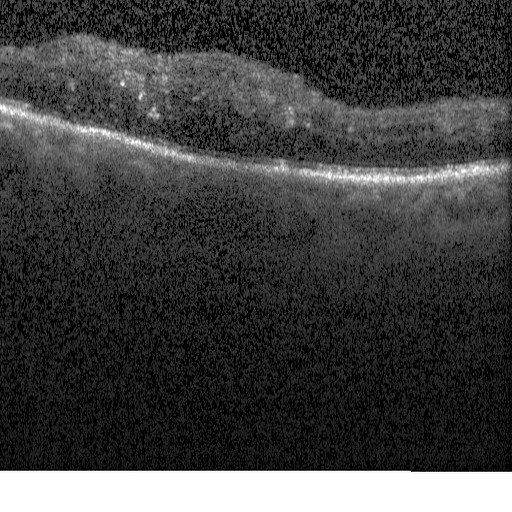
Heidelberg Spectralis, OCT line scan
The scan shows DME.